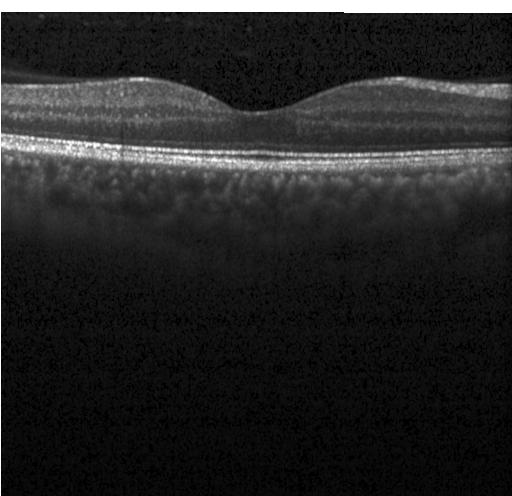

Spectral-domain optical coherence tomography; through the macula; optical coherence tomography B-scan.
Diagnosis: neither choroidal neovascularization, diabetic macular edema, nor drusen.